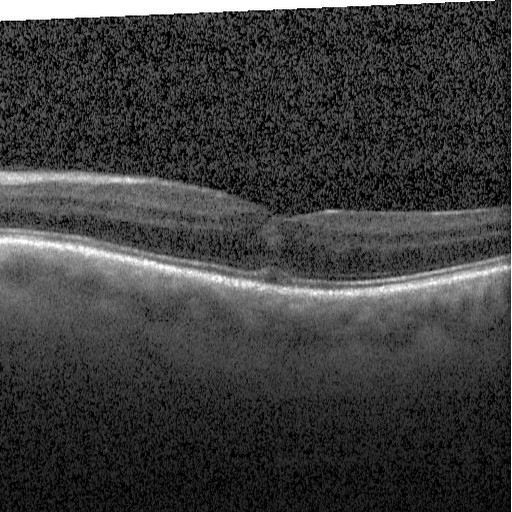

Retinal OCT B-scan · SD-OCT. Impression: DME.